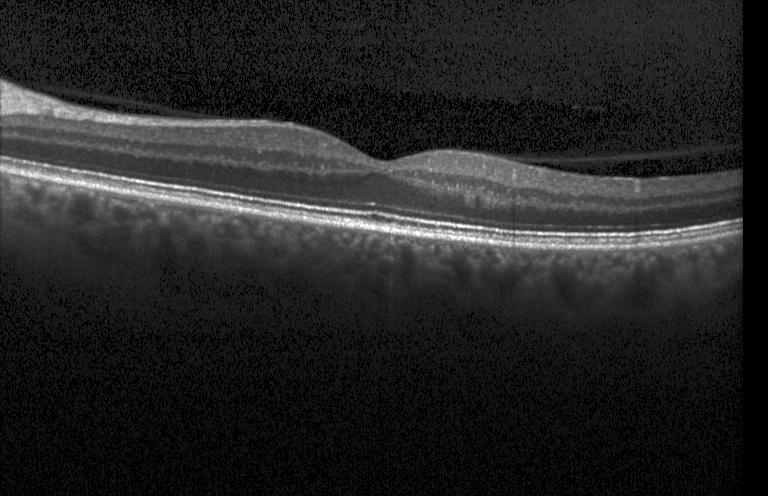
Diagnosis: no choroidal neovascularization, diabetic macular edema, or drusen.